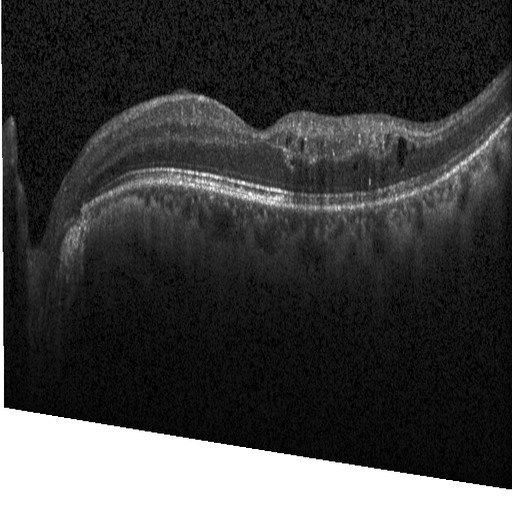

Retinal OCT B-scan. Spectral-domain OCT.
The scan shows diabetic macular edema.